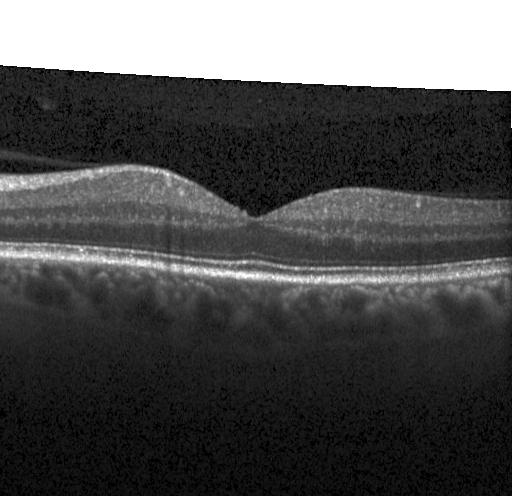

Impression: no choroidal neovascularization, diabetic macular edema, or drusen.